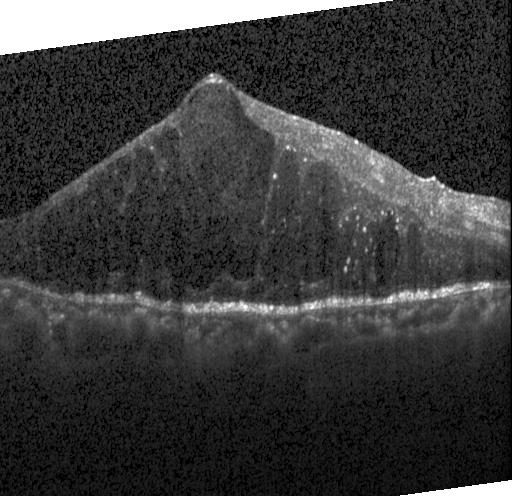 Impression: diabetic macular edema.